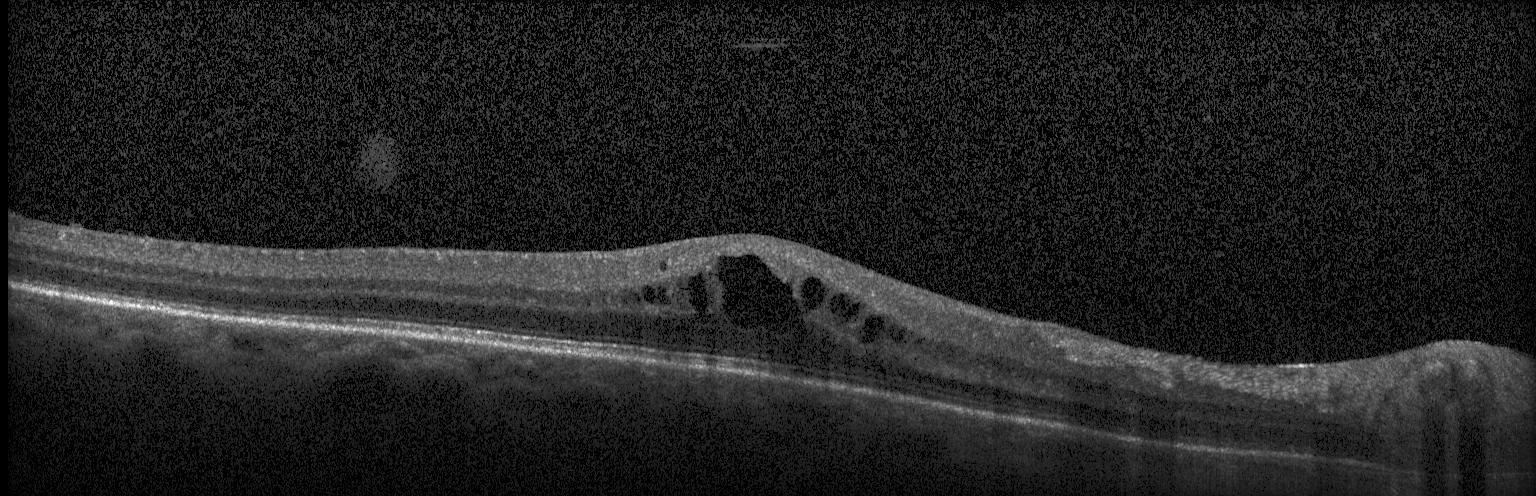

Retinal OCT B-scan, acquired on a Heidelberg Spectralis, SD-OCT — This B-scan demonstrates diabetic macular edema.